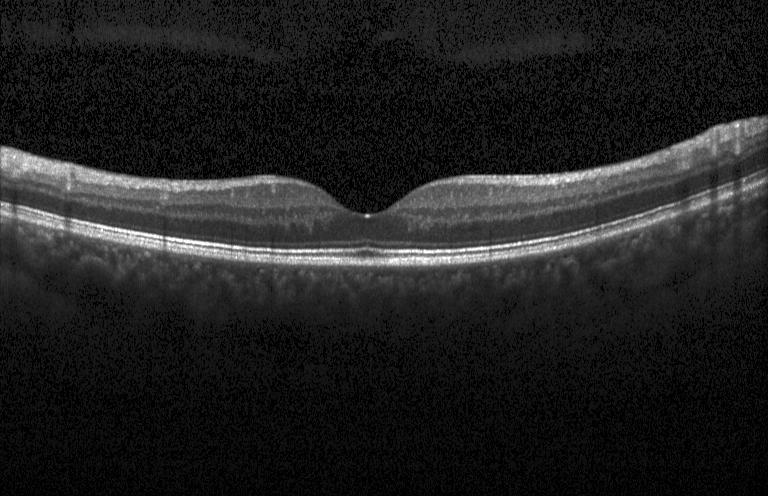

The scan shows neither choroidal neovascularization, diabetic macular edema, nor drusen.